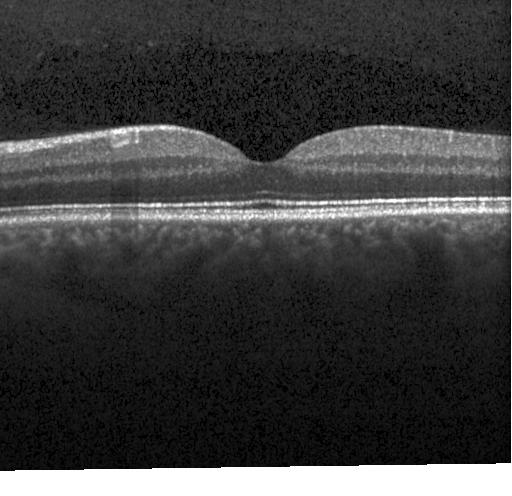
Retinal OCT cross-section showing no evidence of choroidal neovascularization, diabetic macular edema, or drusen.